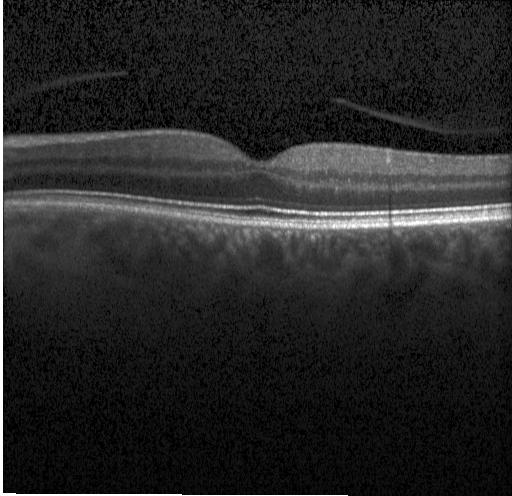

Spectral-domain OCT B-scan: no CNV, DME, or drusen.